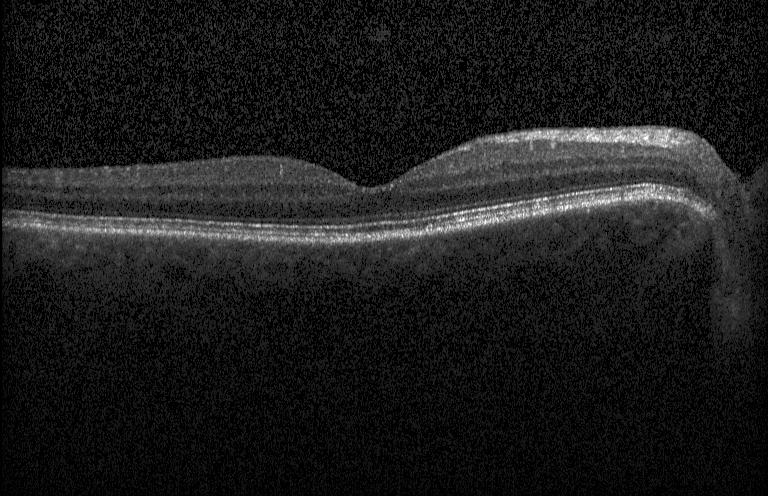

Optical coherence tomography B-scan. Spectral-domain optical coherence tomography
The scan shows no choroidal neovascularization, no diabetic macular edema, and no drusen.